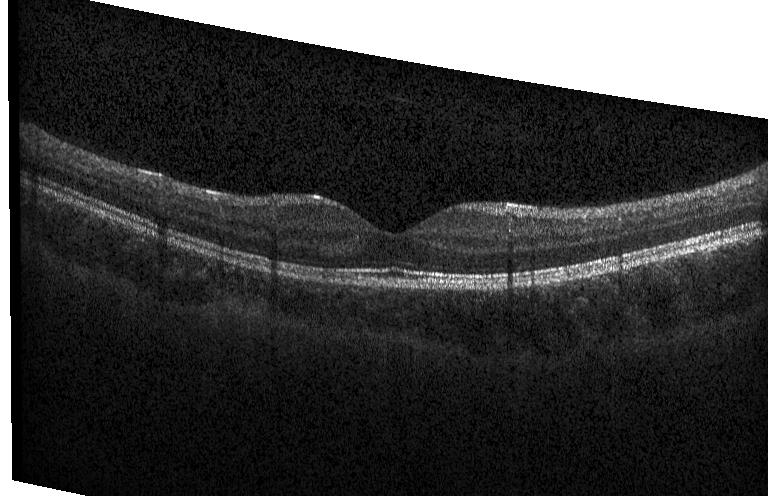
OCT scan showing no choroidal neovascularization, diabetic macular edema, or drusen.